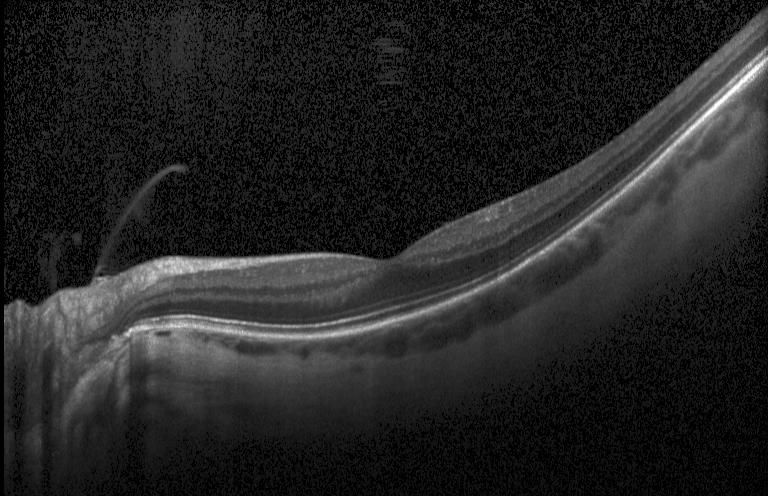 Heidelberg Spectralis OCT system; spectral-domain optical coherence tomography; optical coherence tomography B-scan — No CNV, DME, or drusen.